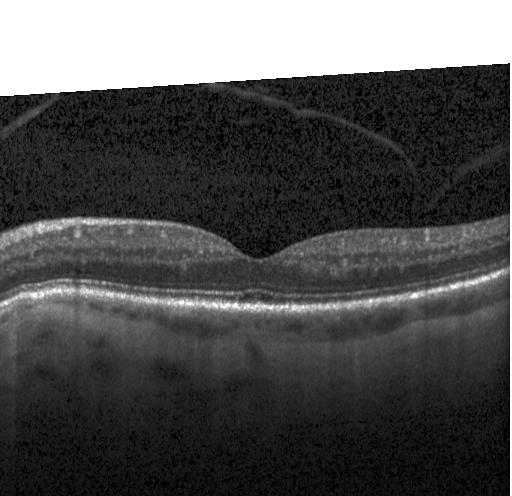

Horizontal scan through the fovea; retinal OCT B-scan
OCT finding: no CNV, DME, or drusen.